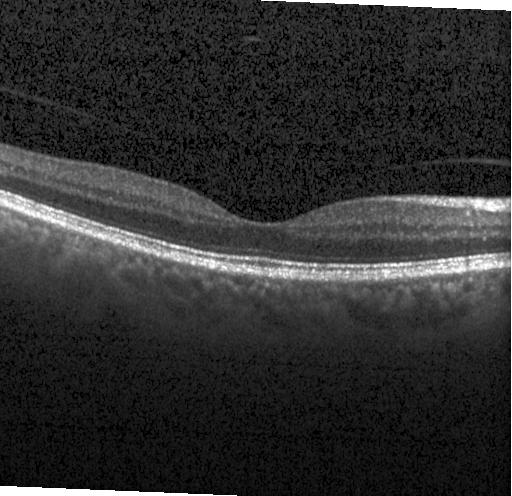
Diagnosis: no choroidal neovascularization, no diabetic macular edema, and no drusen.